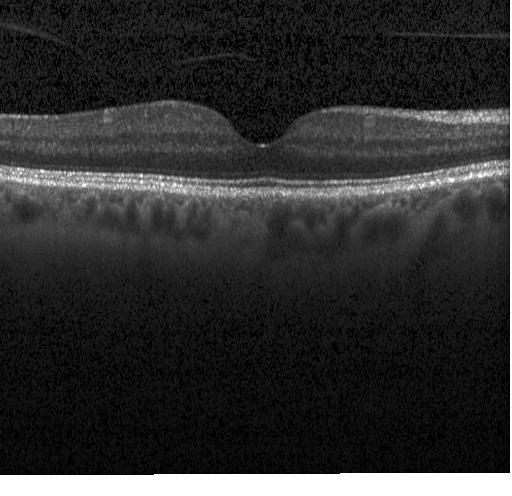

Retinal OCT cross-section — Diagnosis: no choroidal neovascularization, no diabetic macular edema, and no drusen.